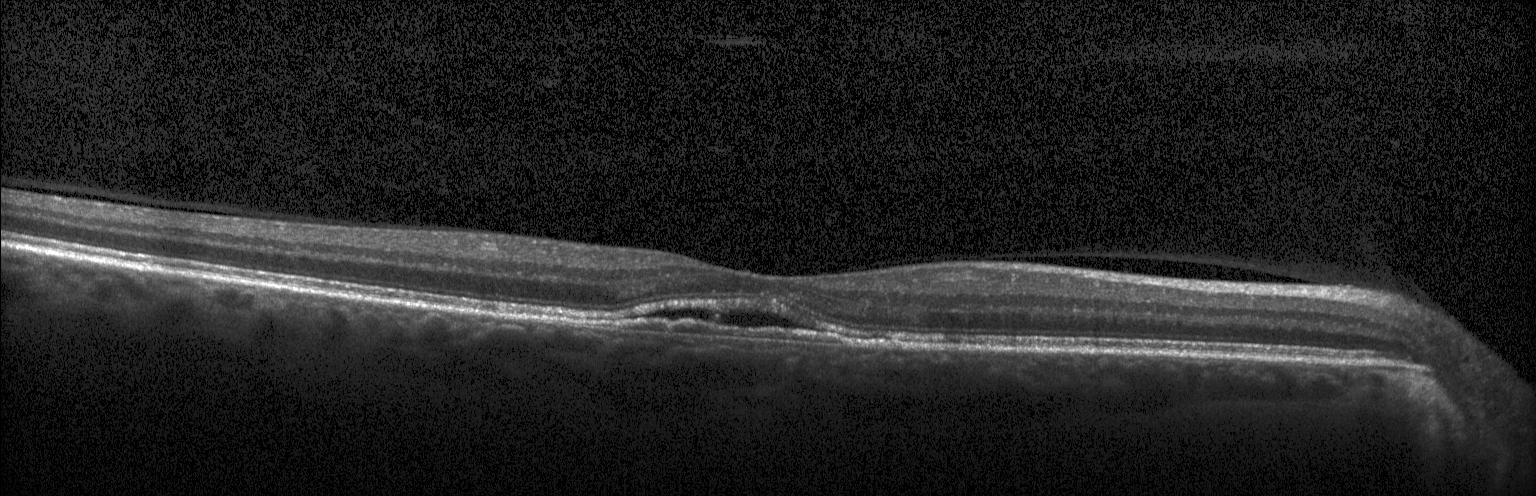
Heidelberg Spectralis OCT system; optical coherence tomography scan
Impression: choroidal neovascularization.